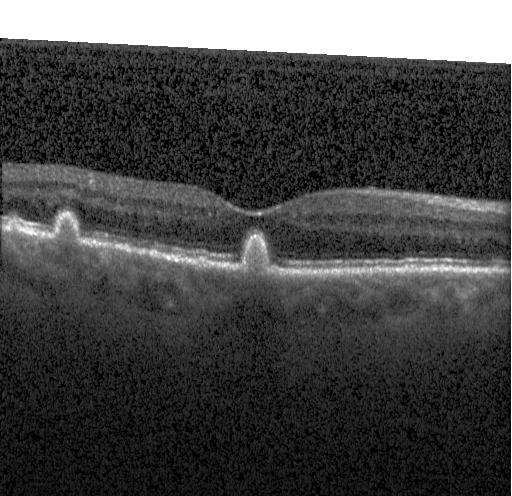

Centered on the fovea · spectral-domain optical coherence tomography · retinal OCT B-scan — Assessment: sub-RPE drusenoid deposits.